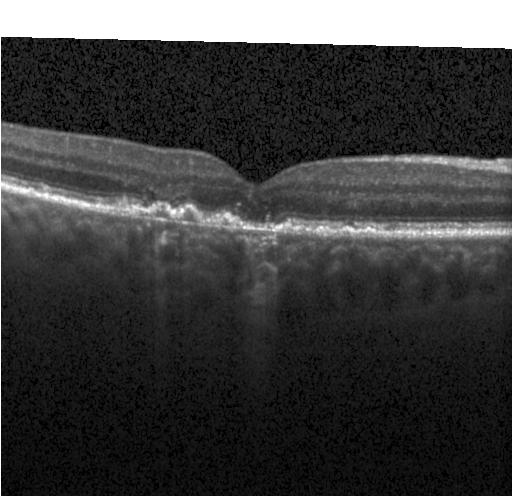
Optical coherence tomography B-scan; Heidelberg Spectralis OCT system; SD-OCT; fovea-centered
Dx: choroidal neovascularization (CNV).